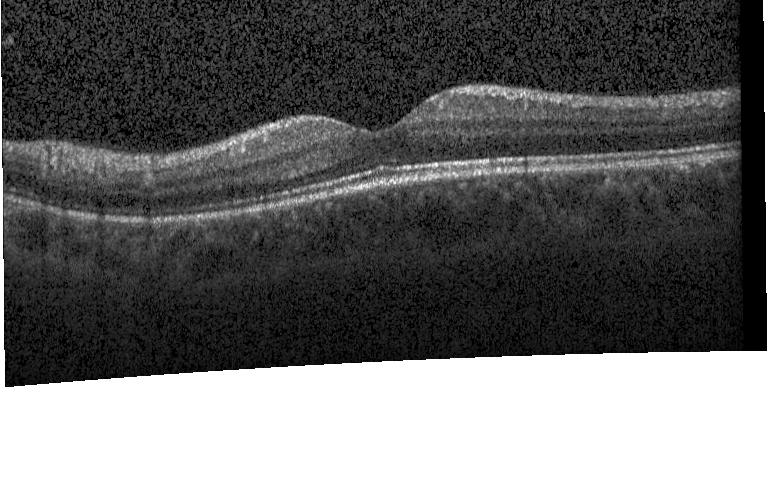 Macular OCT: no choroidal neovascularization, no diabetic macular edema, and no drusen.